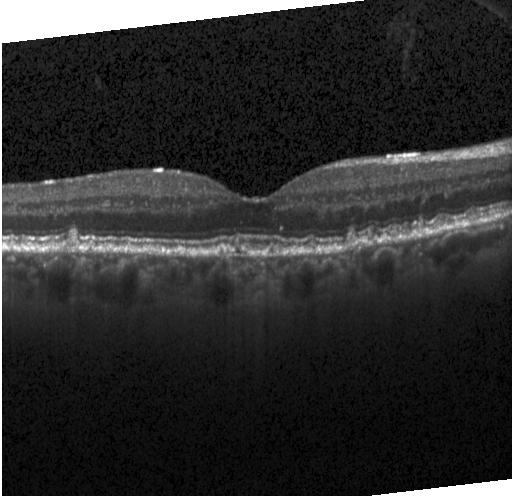
Retinal OCT cross-section, spectral-domain OCT — Drusen.